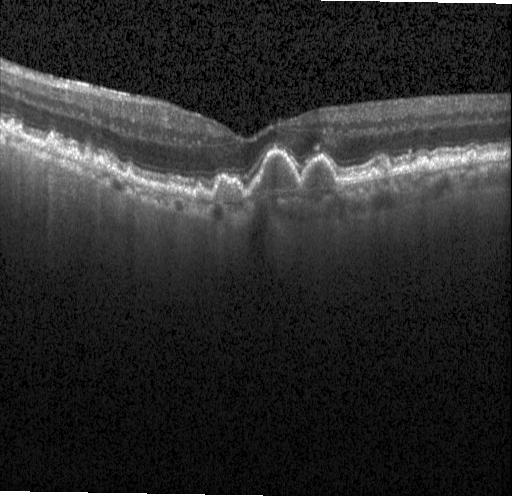
Retinal OCT cross-section · spectral-domain OCT
Impression: multiple drusen.